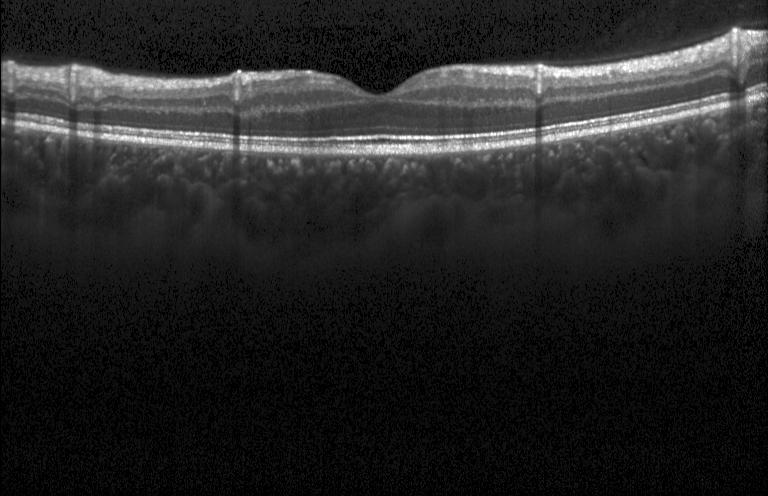
OCT B-scan showing no choroidal neovascularization, diabetic macular edema, or drusen.